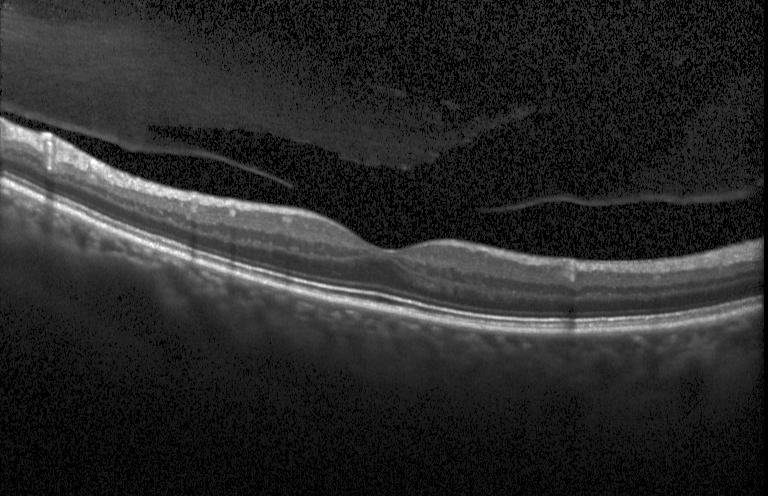

Optical coherence tomography B-scan; spectral-domain OCT — Diagnosis: neither choroidal neovascularization, diabetic macular edema, nor drusen.